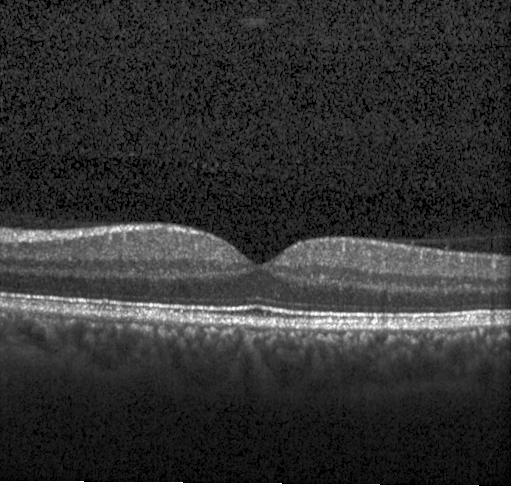

Through the macula · retinal OCT B-scan · Heidelberg Spectralis OCT system. The scan shows no evidence of choroidal neovascularization, diabetic macular edema, or drusen.